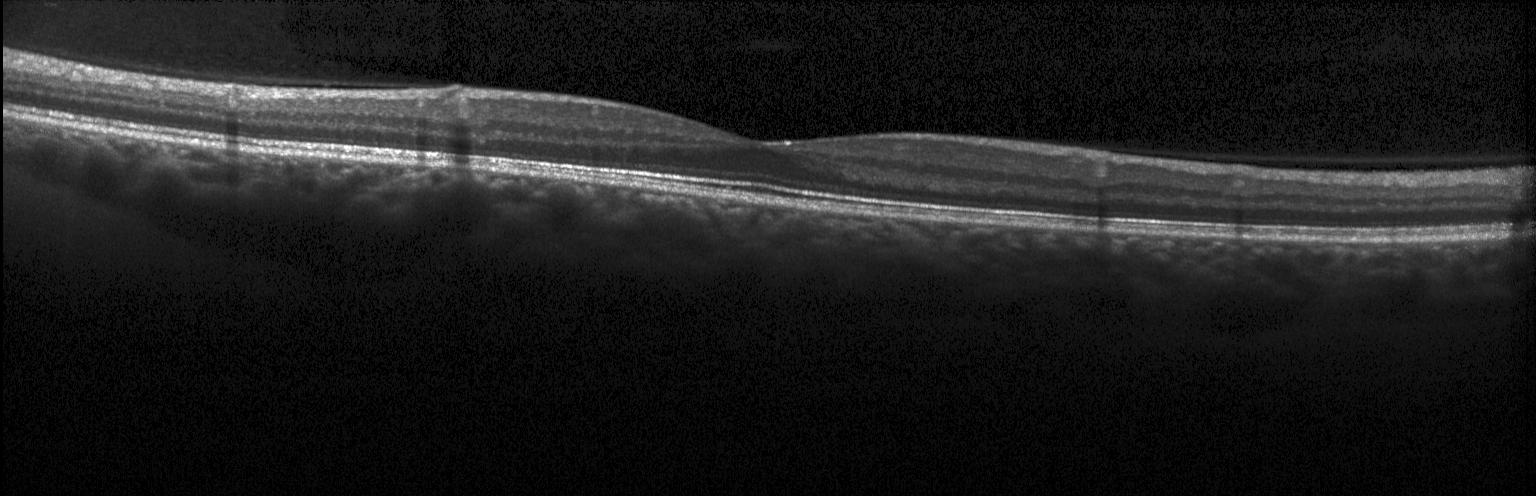
Optical coherence tomography B-scan, centered on the fovea.
Finding: neither choroidal neovascularization, diabetic macular edema, nor drusen.